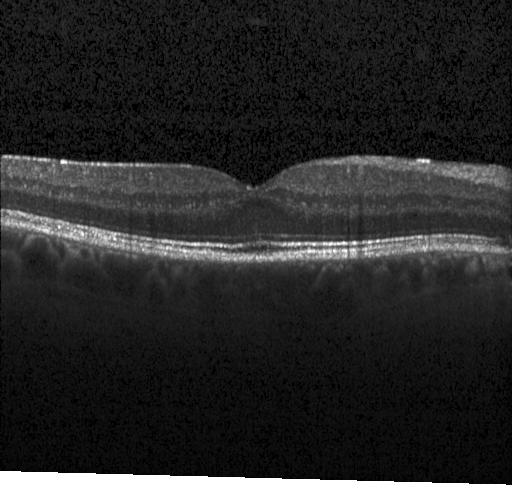
Optical coherence tomography scan — Finding: neither choroidal neovascularization, diabetic macular edema, nor drusen.